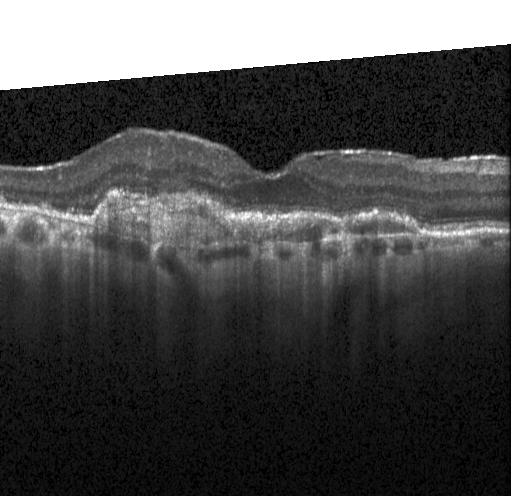

OCT finding: CNV.